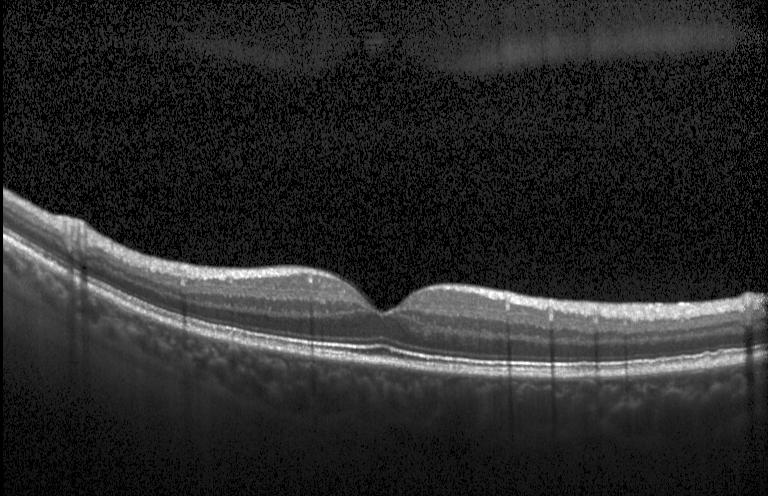

Impression: neither CNV, DME, nor drusen.